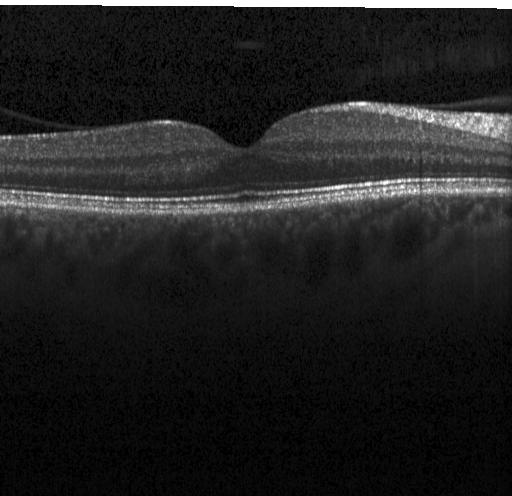 Finding: no CNV, no DME, and no drusen.